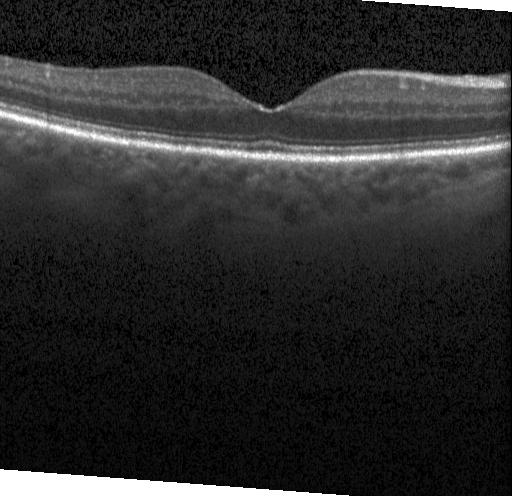

Heidelberg Spectralis · fovea-centered · optical coherence tomography scan
Impression: neither choroidal neovascularization, diabetic macular edema, nor drusen.